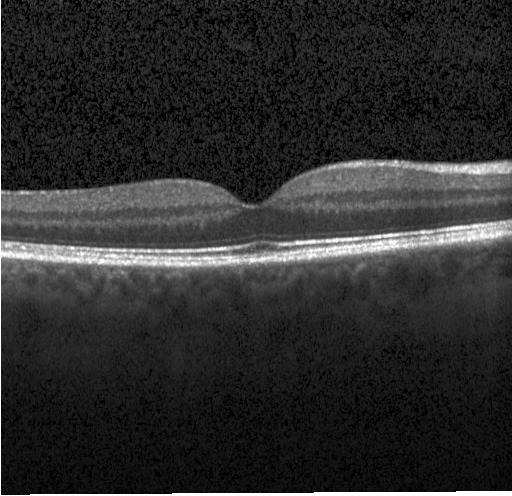 Retinal OCT B-scan, spectral-domain optical coherence tomography, fovea-centered, acquired on a Heidelberg Spectralis — The scan shows no CNV, DME, or drusen.